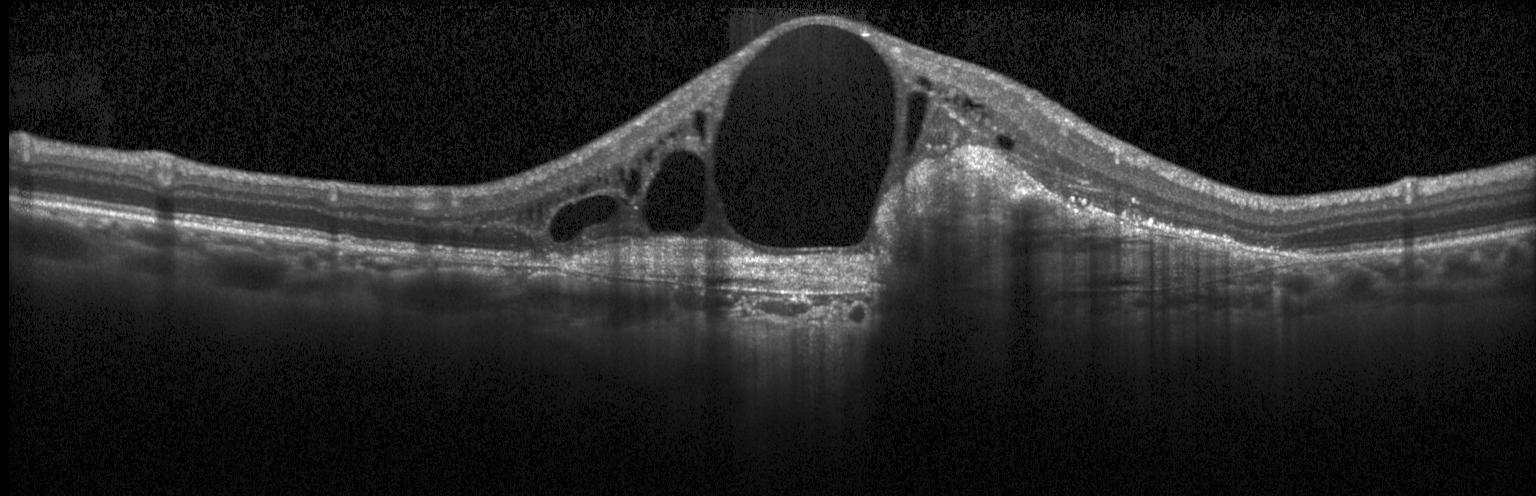

SD-OCT · horizontal scan through the fovea · acquired on a Heidelberg Spectralis · optical coherence tomography B-scan — OCT finding: a choroidal neovascular membrane.